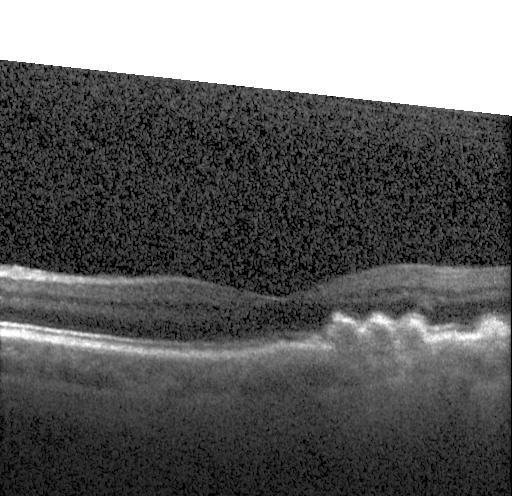
Through the macula; Heidelberg Spectralis OCT system; optical coherence tomography B-scan; spectral-domain optical coherence tomography
Drusen.